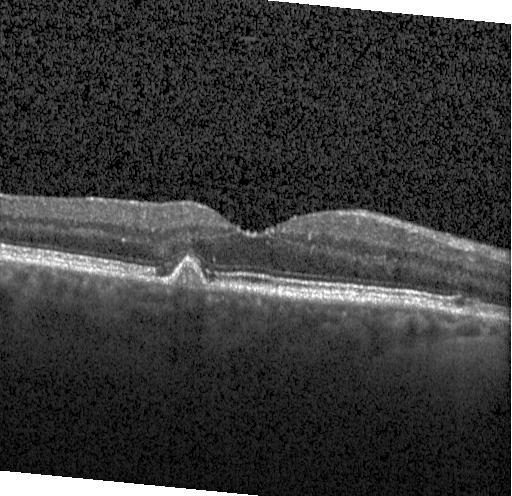

Diagnosis: drusen.